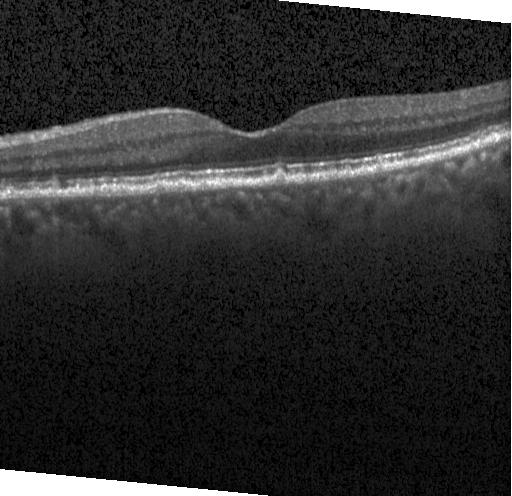 Retinal OCT cross-section, Heidelberg Spectralis OCT system, through the macula, SD-OCT
The scan shows sub-RPE drusenoid deposits.